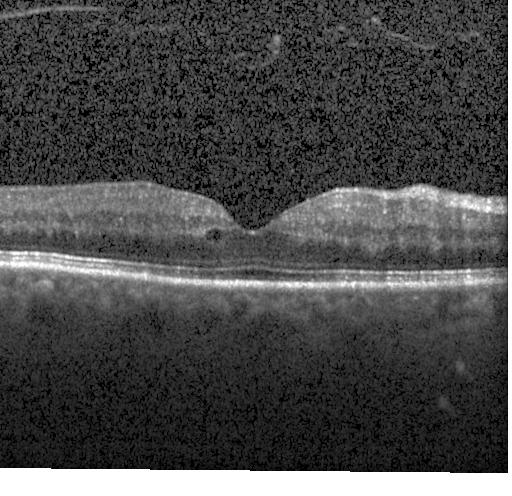

Assessment: DME.